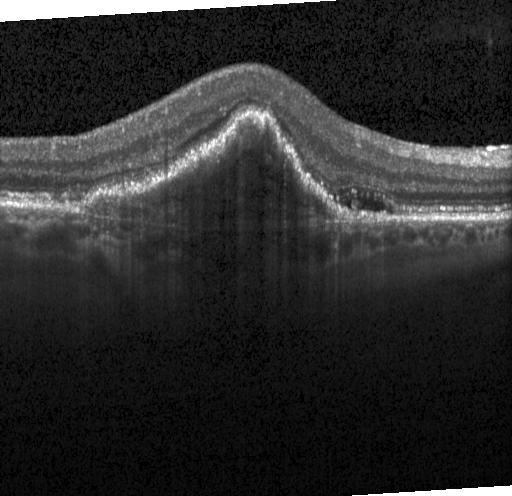
Diagnosis: a choroidal neovascular membrane.